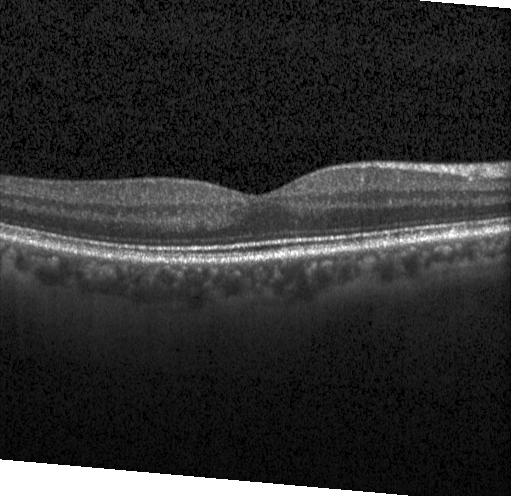

Optical coherence tomography B-scan. SD-OCT. This B-scan demonstrates neither CNV, DME, nor drusen.